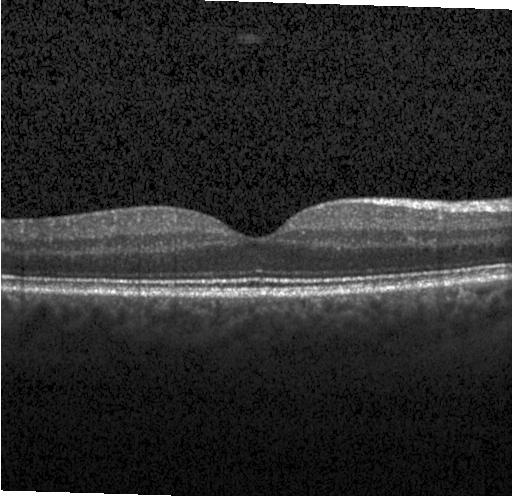

OCT line scan — This B-scan demonstrates no evidence of choroidal neovascularization, diabetic macular edema, or drusen.